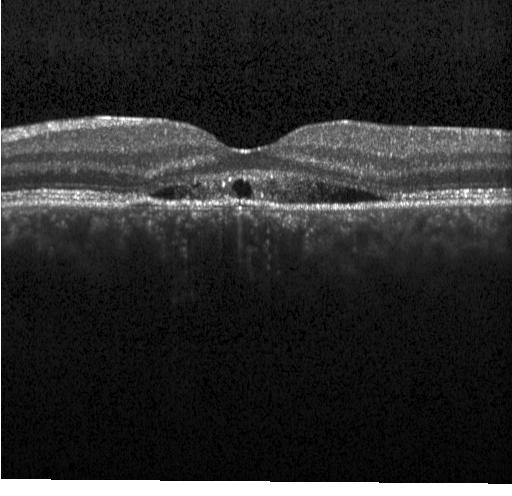
OCT B-scan — This B-scan demonstrates choroidal neovascularization.